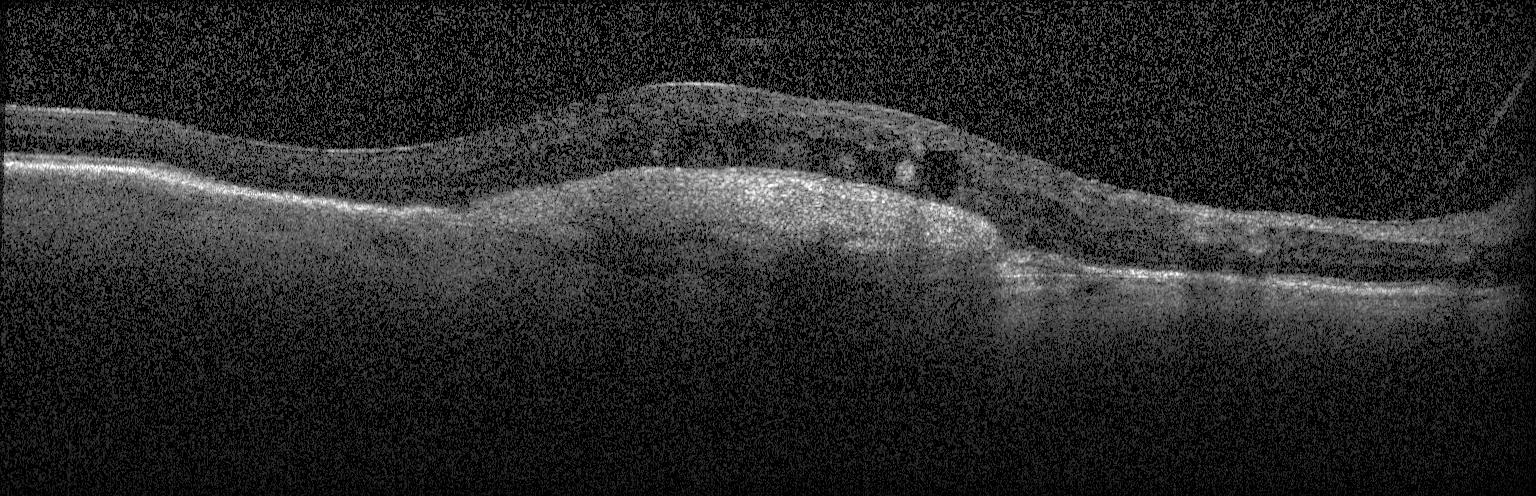 Retinal OCT cross-section, centered on the fovea.
Diagnosis: CNV.